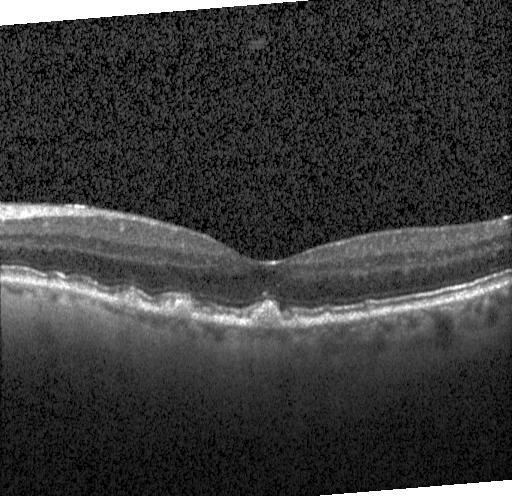

OCT line scan. Heidelberg Spectralis OCT system — Diagnosis: multiple drusen.